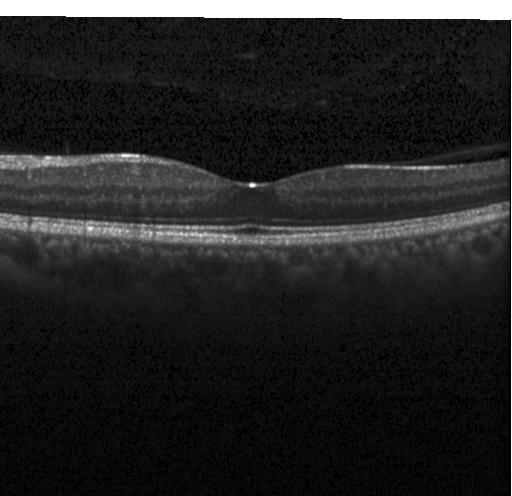

Macular OCT demonstrating no evidence of CNV, DME, or drusen.